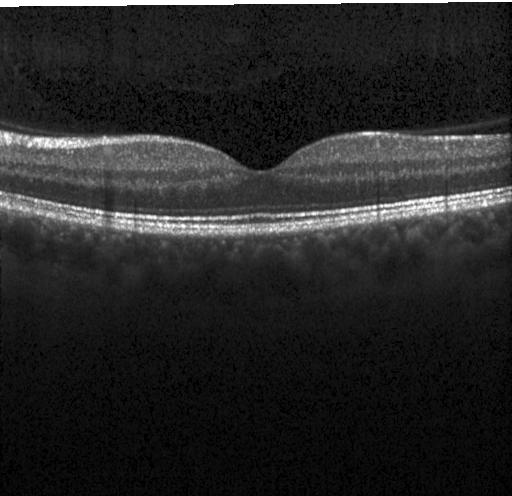

Finding: no CNV, DME, or drusen.